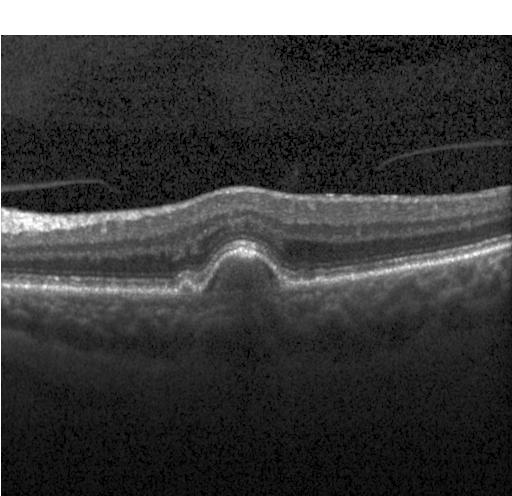

Retinal OCT cross-section; spectral-domain OCT. The scan shows choroidal neovascularization.